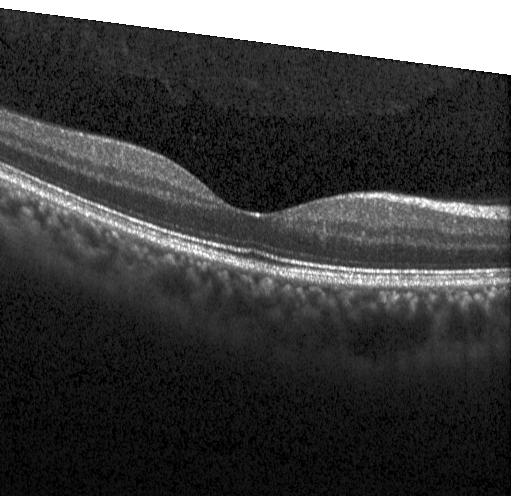 No evidence of CNV, DME, or drusen.